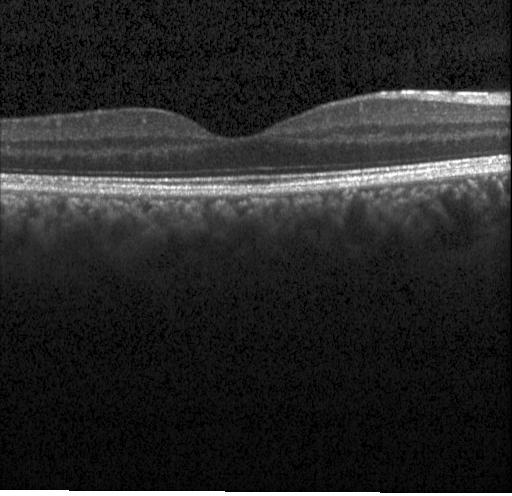 Spectral-domain OCT B-scan: no choroidal neovascularization, no diabetic macular edema, and no drusen.